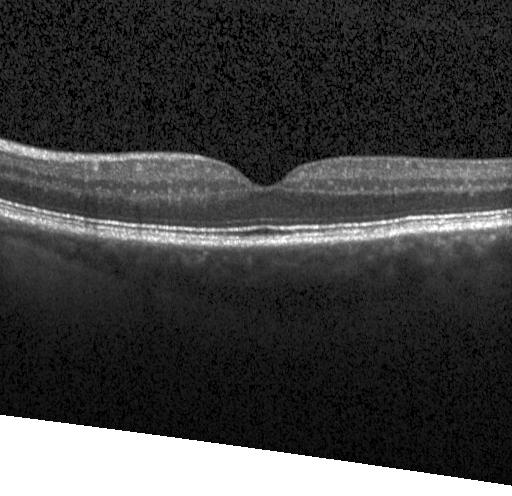 OCT finding: no choroidal neovascularization, no diabetic macular edema, and no drusen.